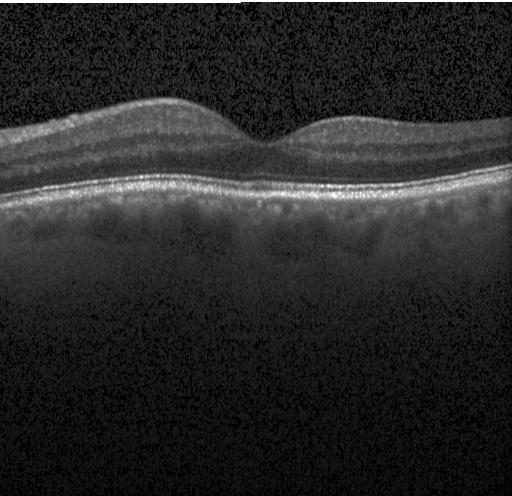
Spectral-domain optical coherence tomography, macular scan, acquired on a Heidelberg Spectralis, optical coherence tomography B-scan. Dx: neither choroidal neovascularization, diabetic macular edema, nor drusen.